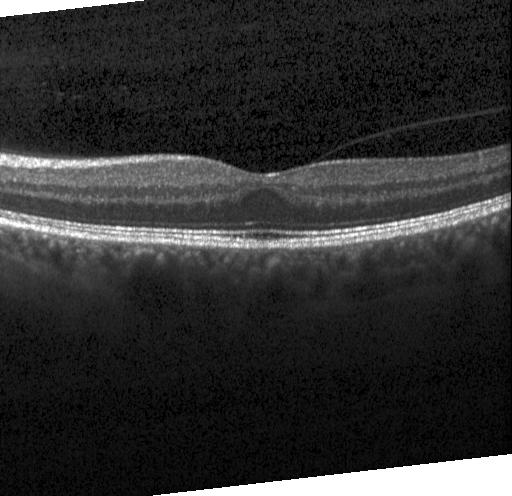 This B-scan demonstrates neither choroidal neovascularization, diabetic macular edema, nor drusen.